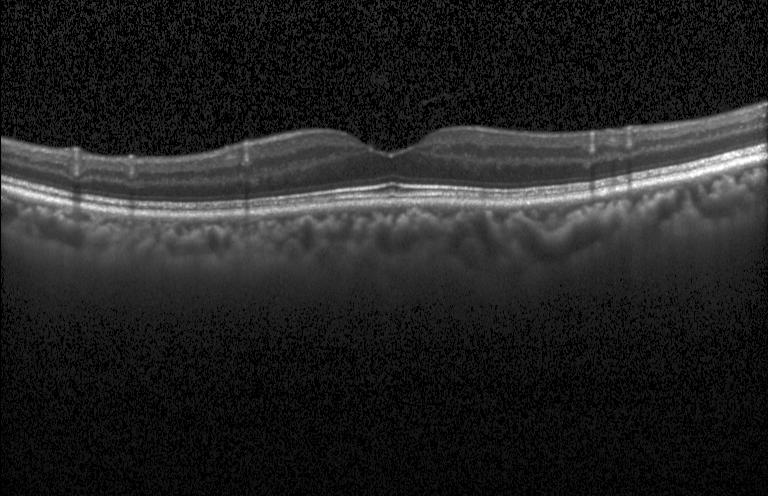

Diagnosis: no evidence of CNV, DME, or drusen.